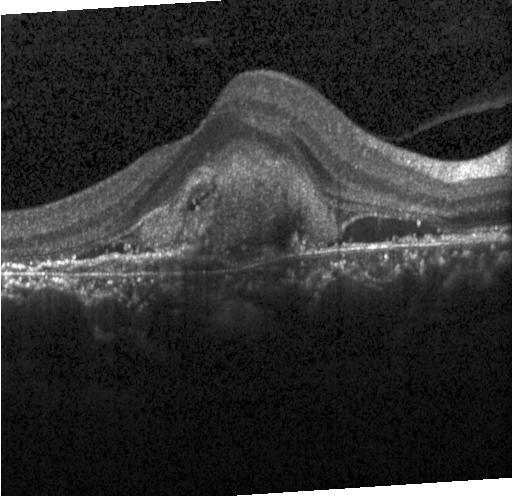

Impression: a choroidal neovascular membrane.